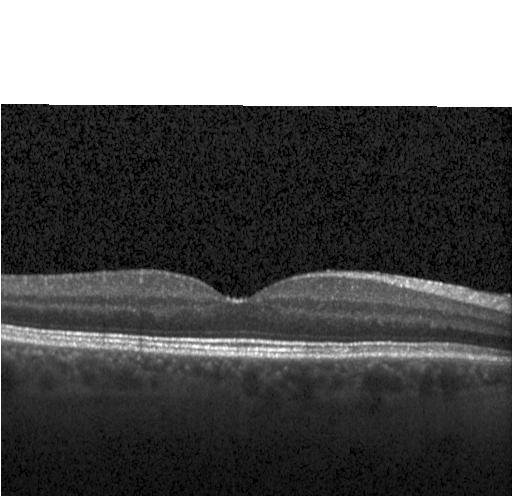 Optical coherence tomography B-scan · Heidelberg Spectralis.
The scan shows neither CNV, DME, nor drusen.